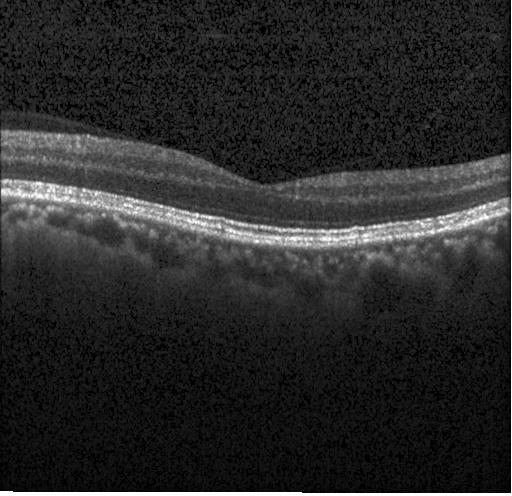 Instrument: Heidelberg Spectralis. OCT B-scan.
Assessment: no CNV, DME, or drusen.